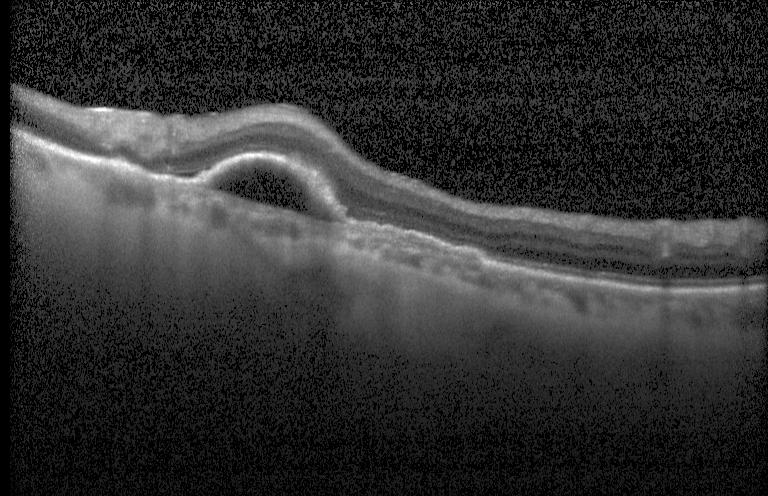 OCT line scan — Dx: CNV.